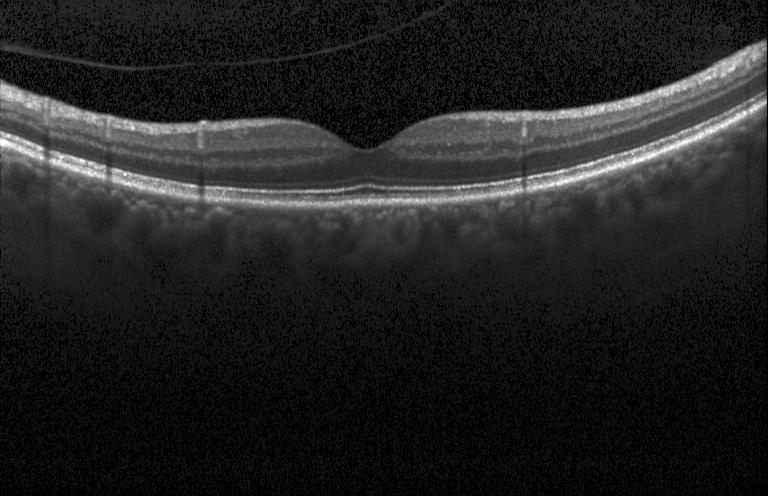

Instrument: Heidelberg Spectralis. Retinal OCT B-scan. Horizontal scan through the fovea. SD-OCT.
Impression: neither CNV, DME, nor drusen.